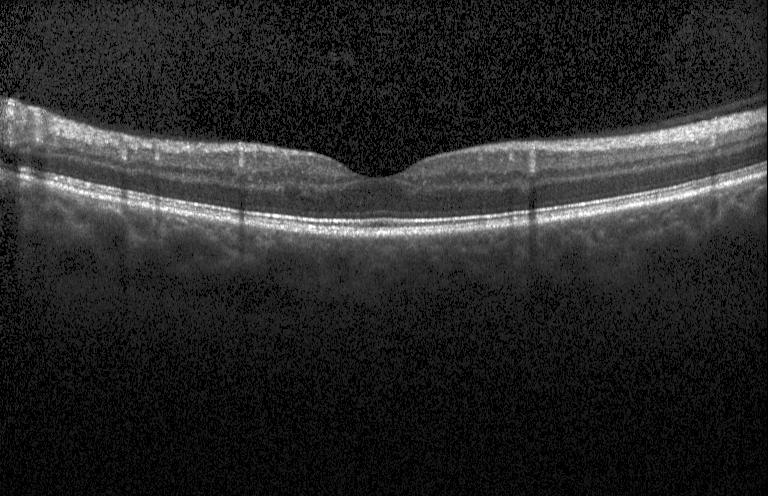 Spectral-domain OCT B-scan: no evidence of CNV, DME, or drusen.